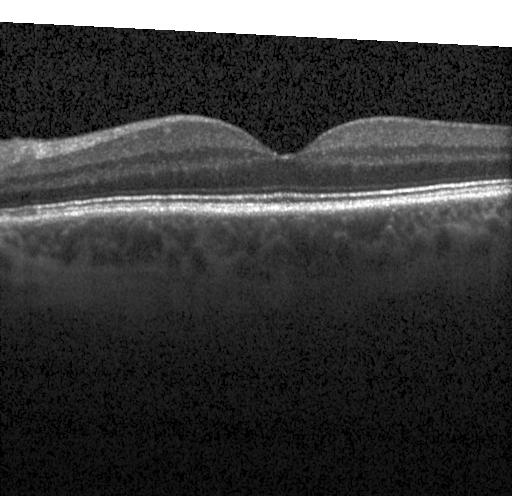

OCT B-scan showing no choroidal neovascularization, no diabetic macular edema, and no drusen.